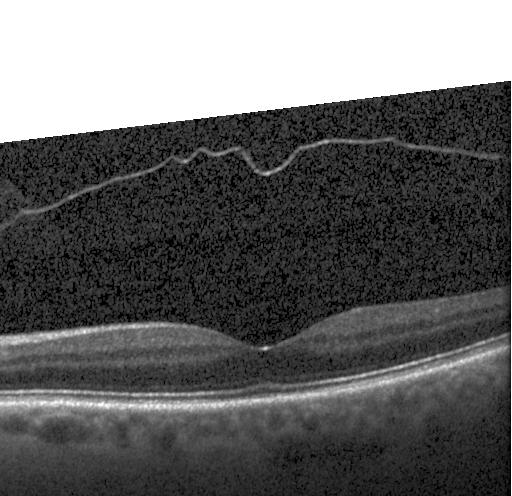
Fovea-centered; SD-OCT; optical coherence tomography B-scan. Finding: no choroidal neovascularization, no diabetic macular edema, and no drusen.